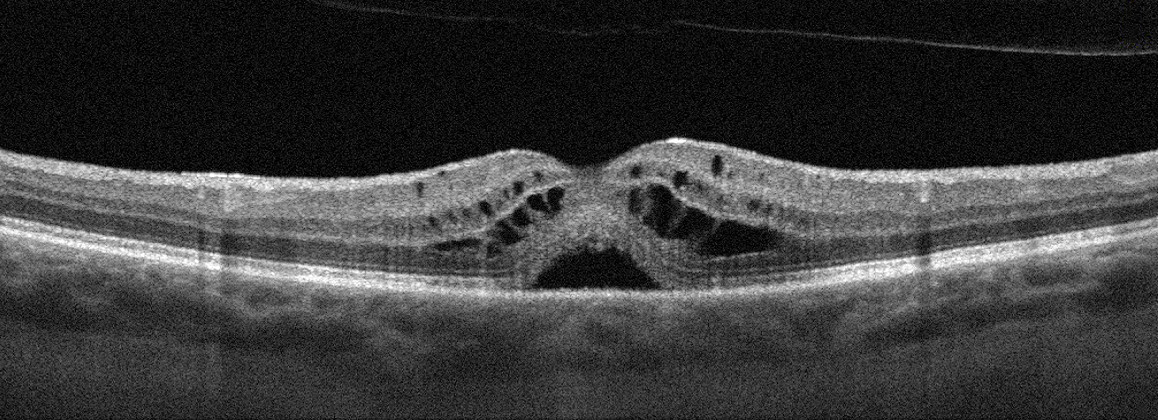 Optovue Avanti RTVue XR; fovea-centered; OCT B-scan — Diagnosis: diabetic macular edema (DME).